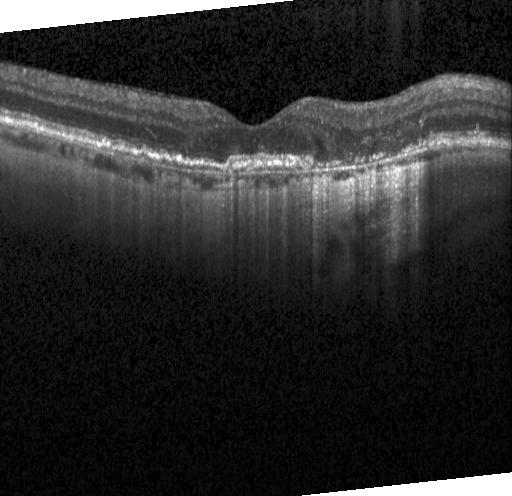
This B-scan demonstrates a choroidal neovascular membrane.